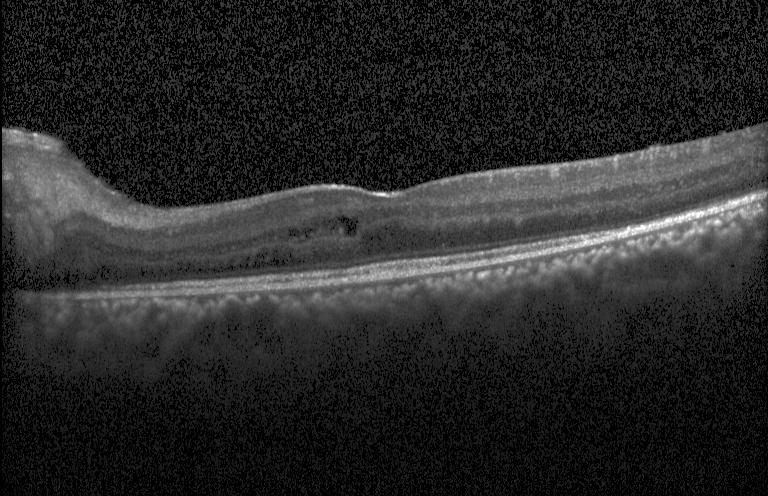
Optical coherence tomography B-scan; SD-OCT; through the macula; Heidelberg Spectralis OCT system.
OCT finding: diabetic macular edema (DME).